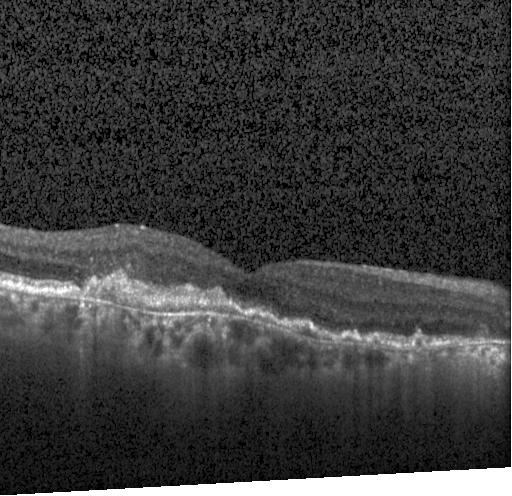
Centered on the fovea; optical coherence tomography scan
A choroidal neovascular membrane.